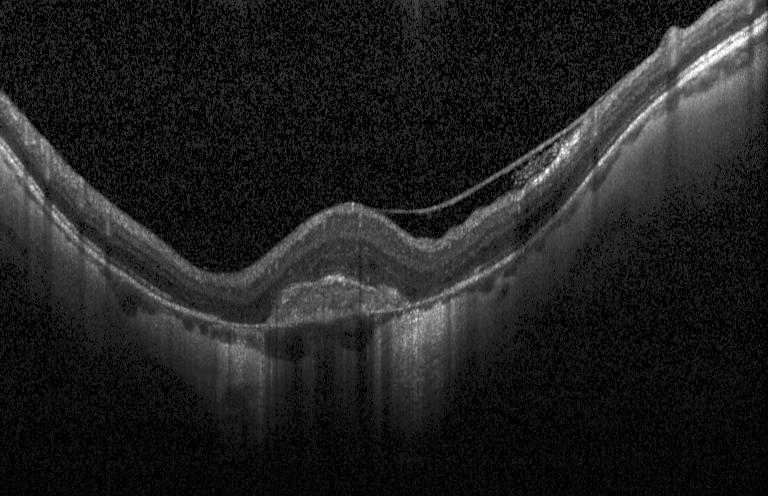
Diagnosis: CNV.